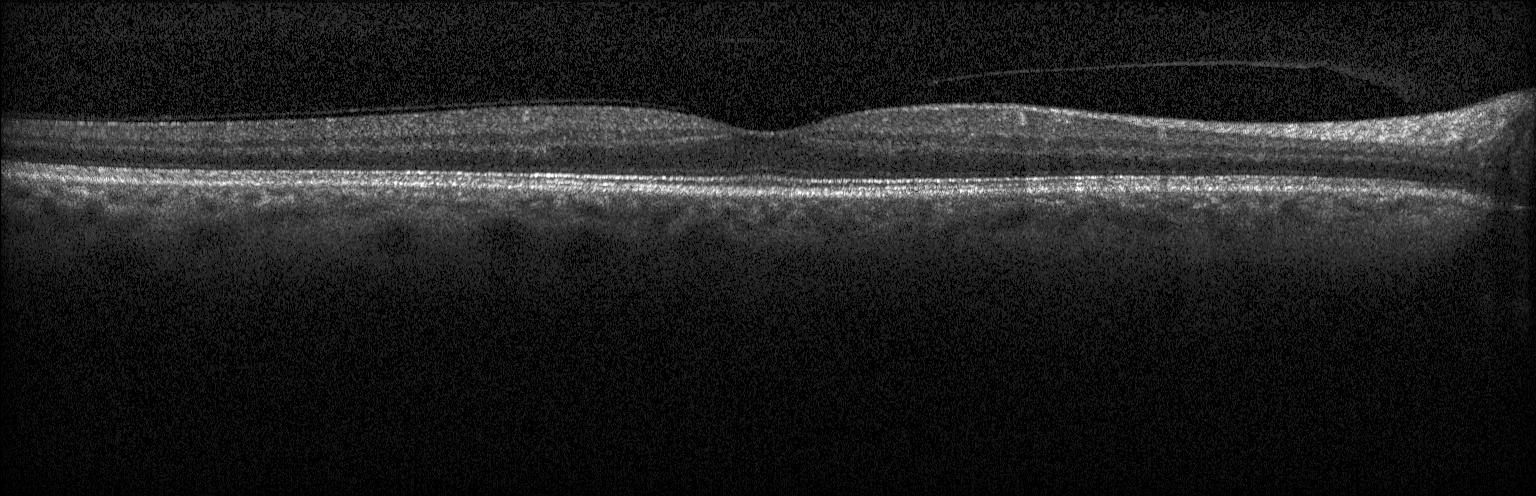
Impression: neither CNV, DME, nor drusen.